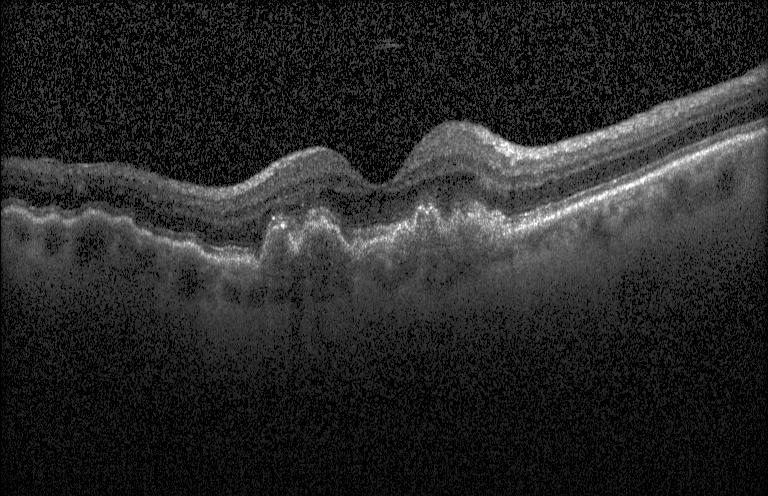

Optical coherence tomography B-scan — A choroidal neovascular membrane.